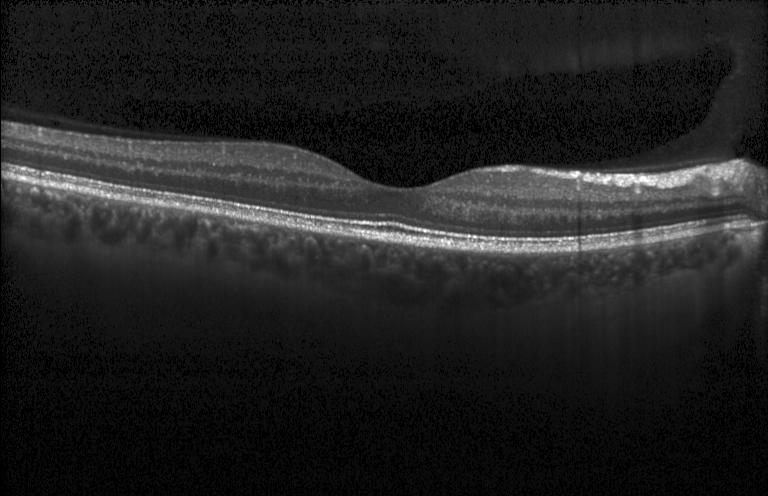

Retinal OCT B-scan, macular scan, Heidelberg Spectralis OCT system
Dx: no CNV, DME, or drusen.